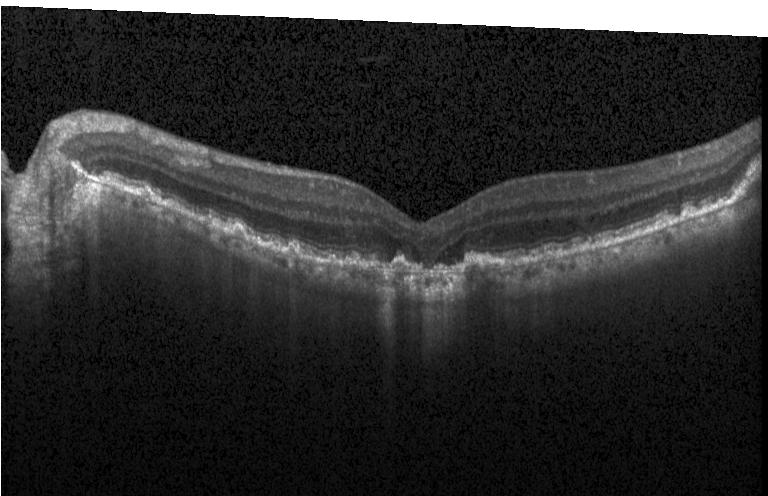

Choroidal neovascularization.